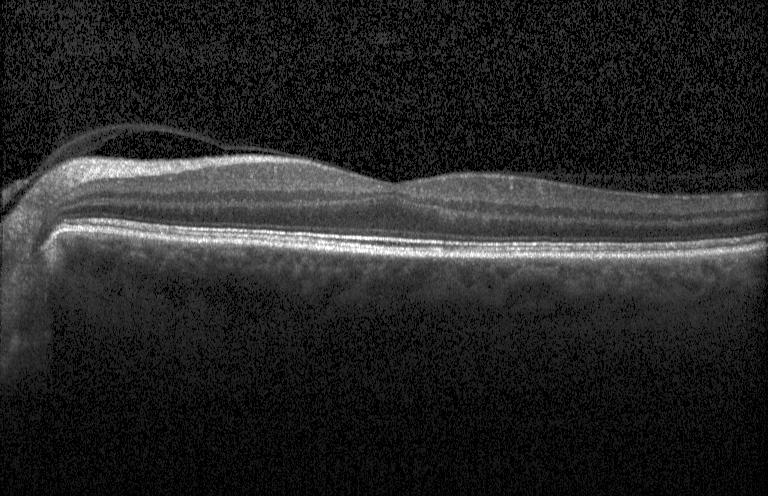

Macular OCT: no CNV, no DME, and no drusen.